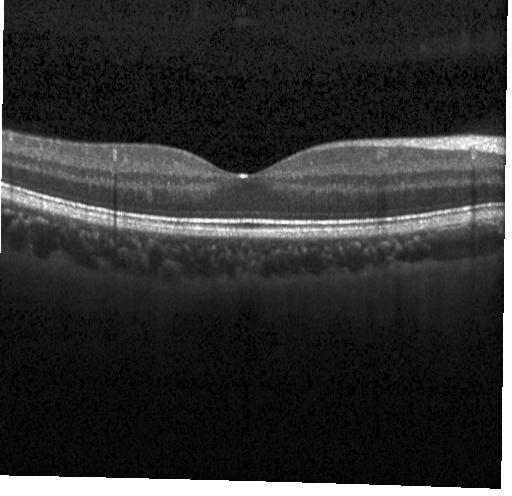
Impression: neither CNV, DME, nor drusen.